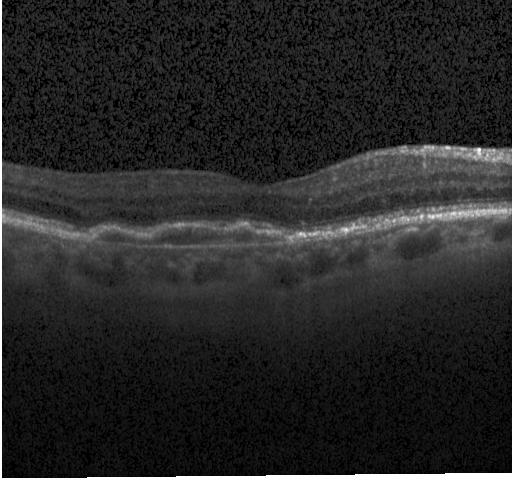

Optical coherence tomography scan, fovea-centered, instrument: Heidelberg Spectralis, spectral-domain OCT. Impression: a choroidal neovascular membrane.